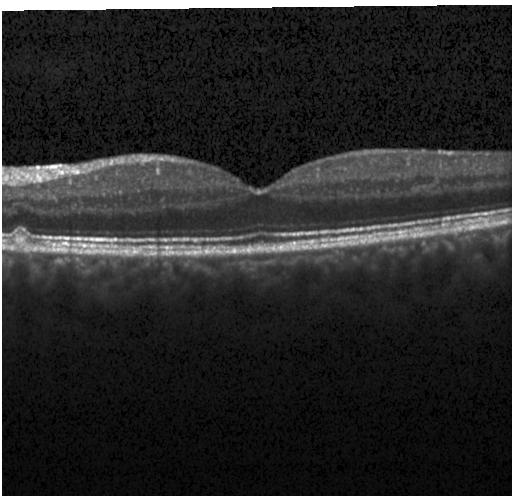

OCT B-scan; spectral-domain OCT; macular scan.
Dx: multiple drusen.